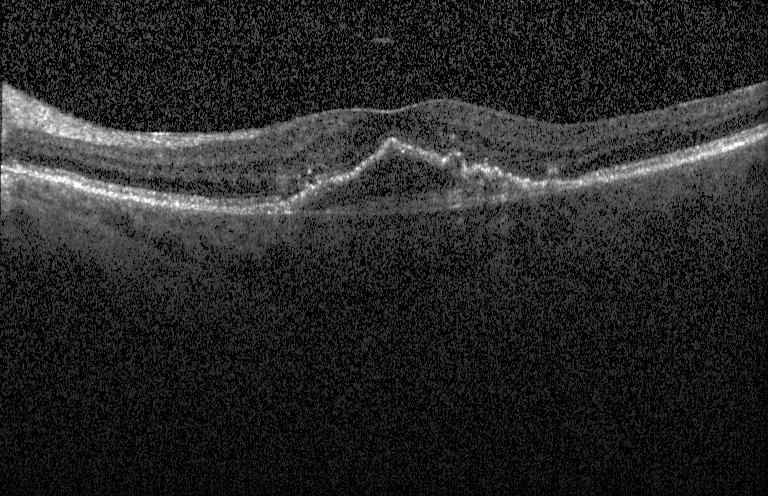
Diagnosis: a choroidal neovascular membrane.